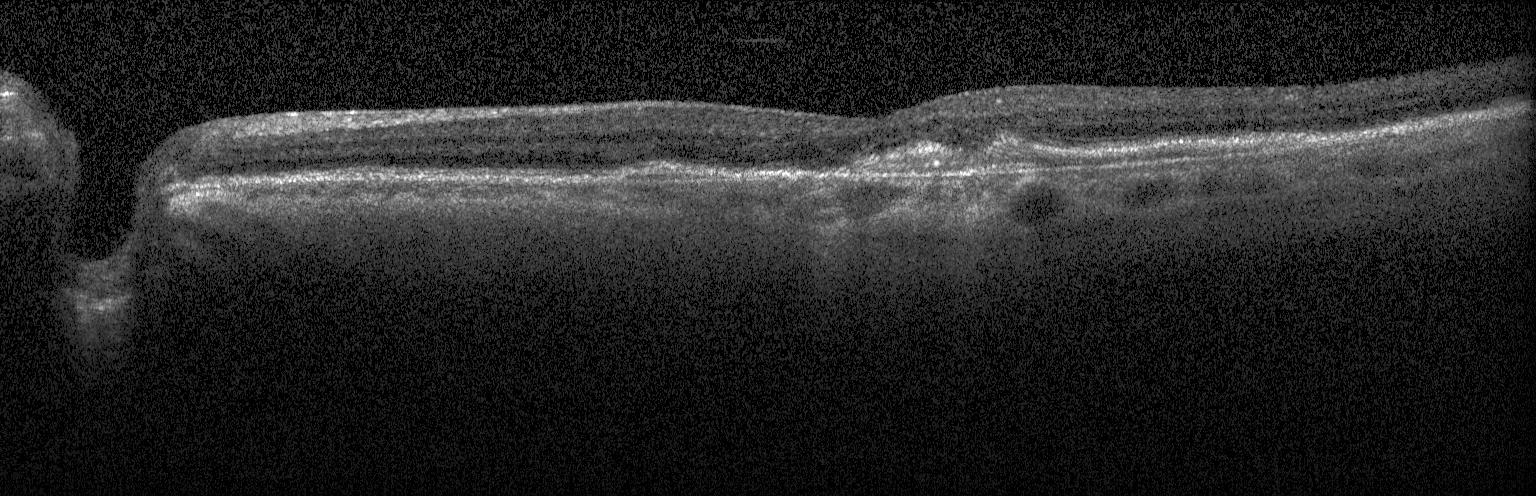

Optical coherence tomography B-scan — This B-scan demonstrates a choroidal neovascular membrane.